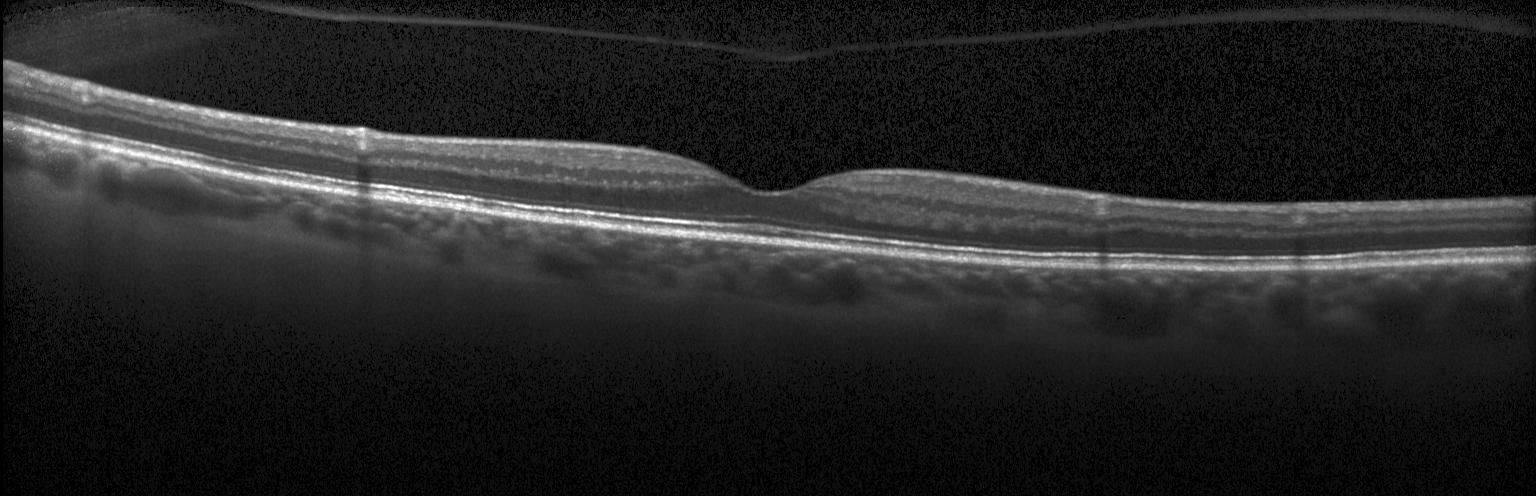 Macular OCT demonstrating neither choroidal neovascularization, diabetic macular edema, nor drusen.